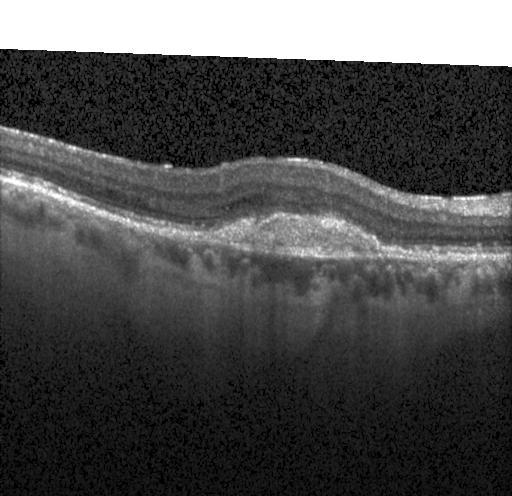 Assessment: a choroidal neovascular membrane.